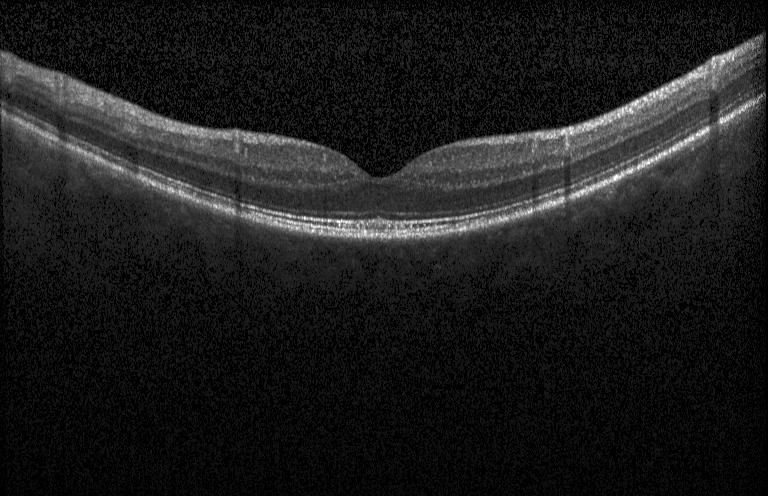

OCT B-scan · spectral-domain optical coherence tomography.
Finding: no choroidal neovascularization, no diabetic macular edema, and no drusen.